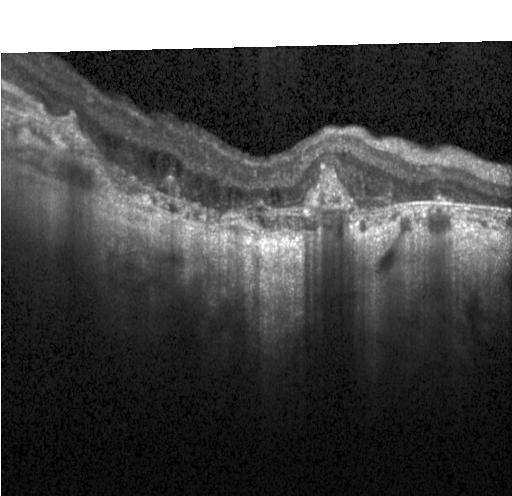

Instrument: Heidelberg Spectralis · centered on the fovea · retinal OCT B-scan.
A choroidal neovascular membrane.